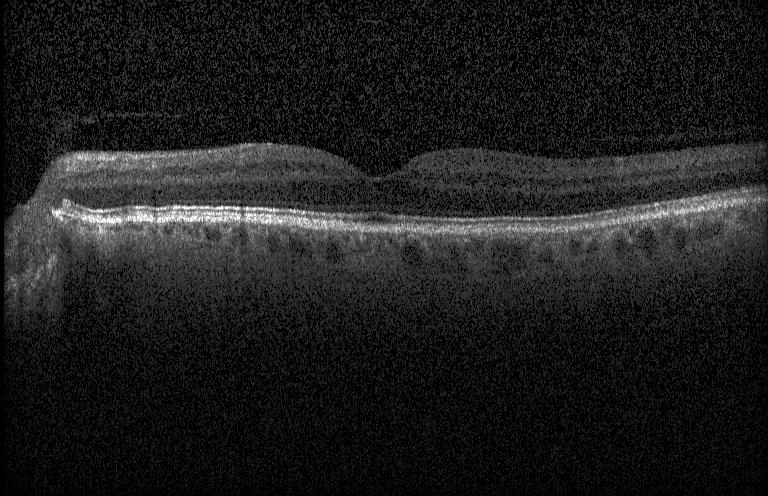

SD-OCT. Retinal OCT cross-section. Diagnosis: no evidence of CNV, DME, or drusen.